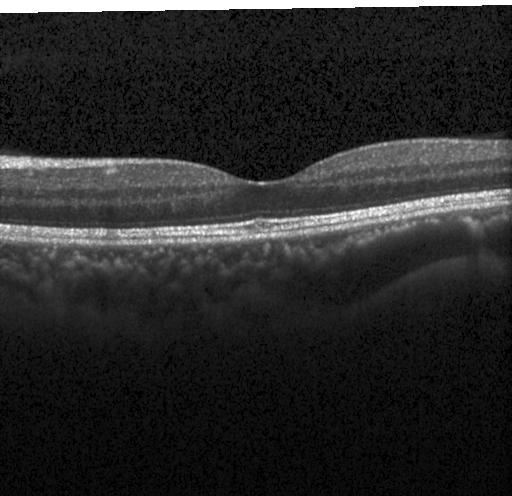 SD-OCT, OCT line scan.
Diagnosis: no evidence of choroidal neovascularization, diabetic macular edema, or drusen.